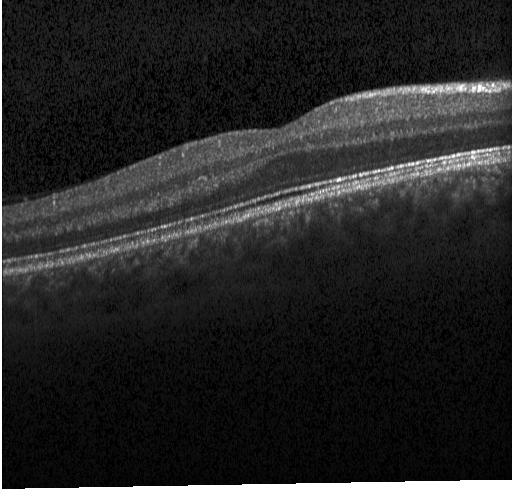
Retinal OCT B-scan.
Dx: no evidence of choroidal neovascularization, diabetic macular edema, or drusen.